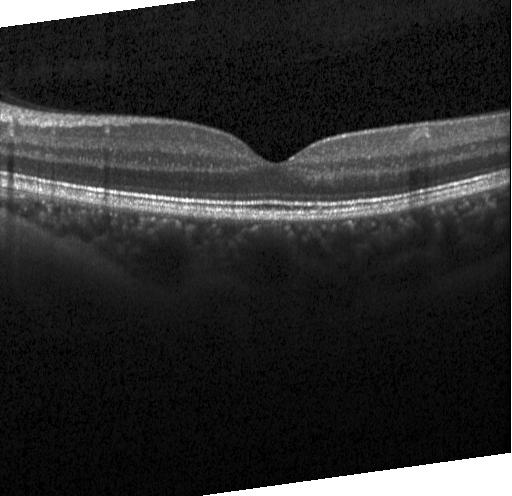

Macular OCT demonstrating no CNV, no DME, and no drusen.